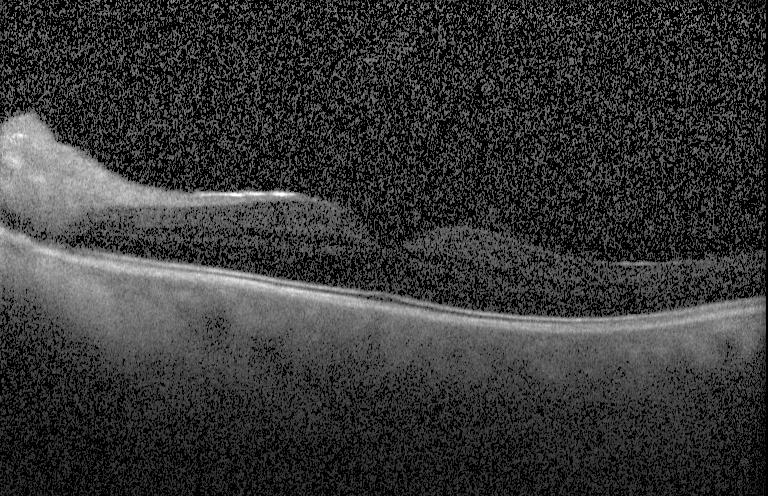 Retinal OCT cross-section, spectral-domain optical coherence tomography, instrument: Heidelberg Spectralis.
Diagnosis: no CNV, DME, or drusen.